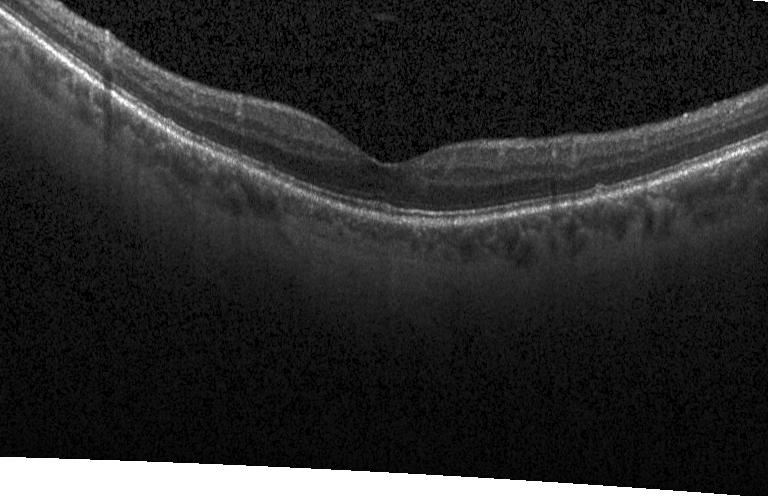

Spectral-domain OCT, horizontal scan through the fovea, Heidelberg Spectralis, optical coherence tomography B-scan
This B-scan demonstrates neither CNV, DME, nor drusen.